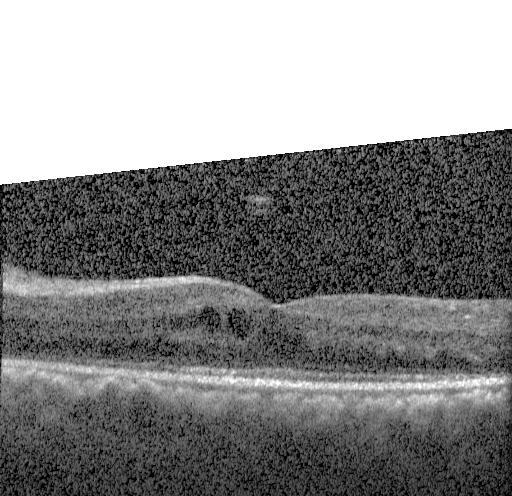
Optical coherence tomography B-scan. Spectral-domain OCT. Macular scan — Assessment: DME.